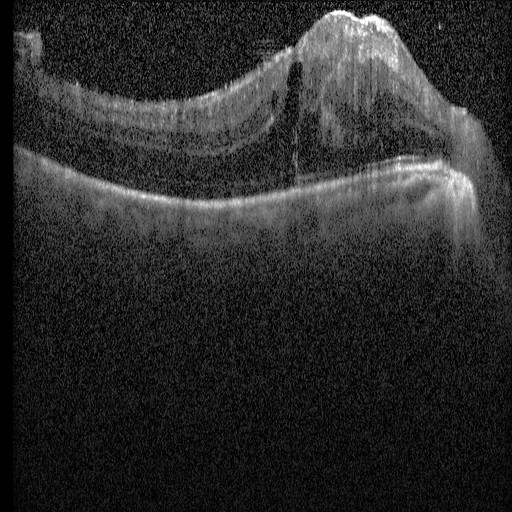
OCT B-scan
Diagnosis: diabetic macular edema (DME).